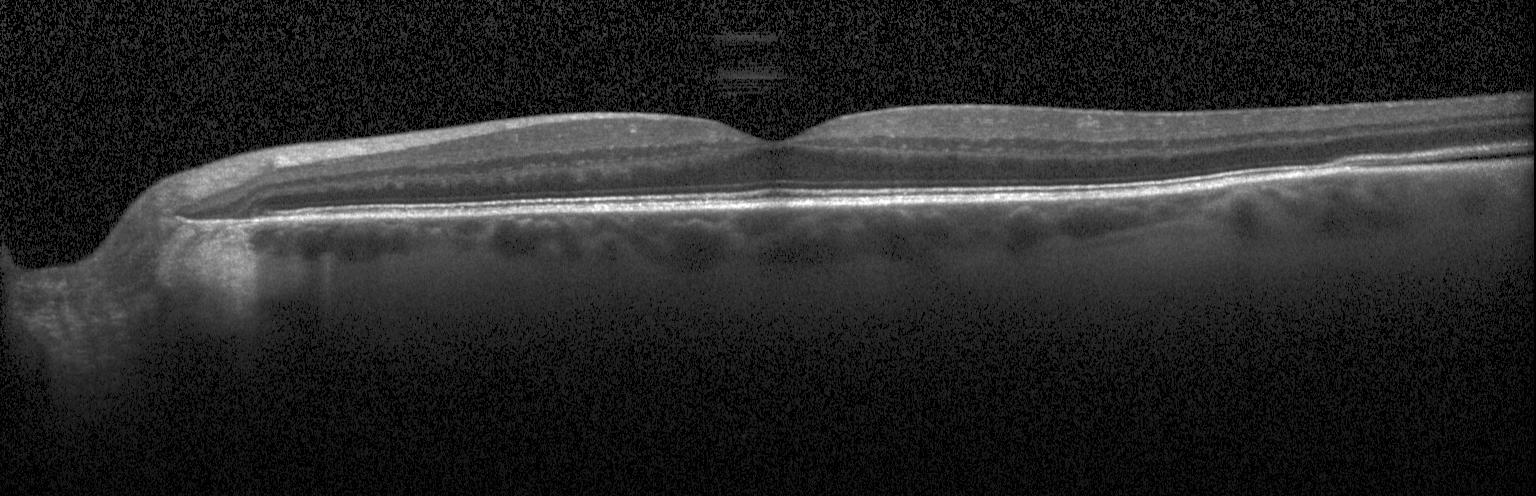
Diagnosis: neither choroidal neovascularization, diabetic macular edema, nor drusen.